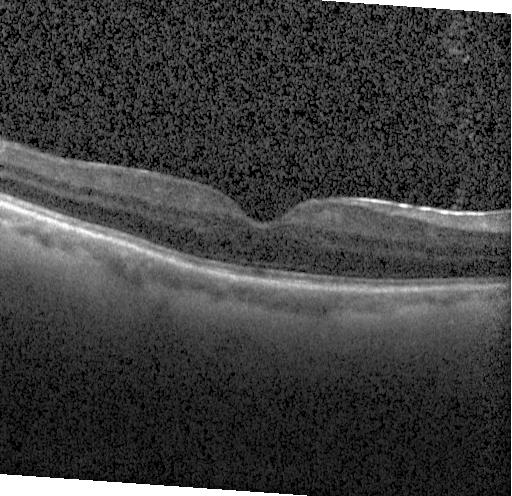
Diagnosis: neither choroidal neovascularization, diabetic macular edema, nor drusen.